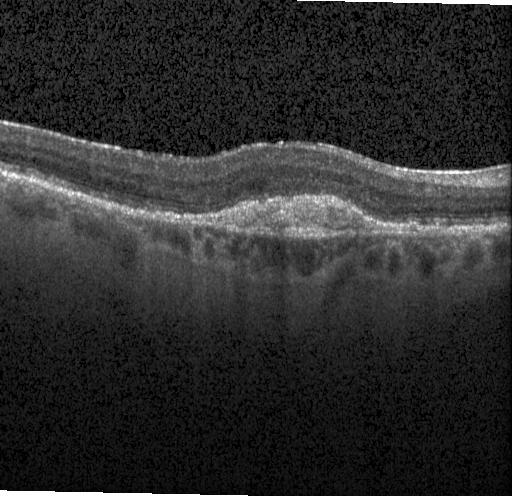
OCT B-scan showing a choroidal neovascular membrane.